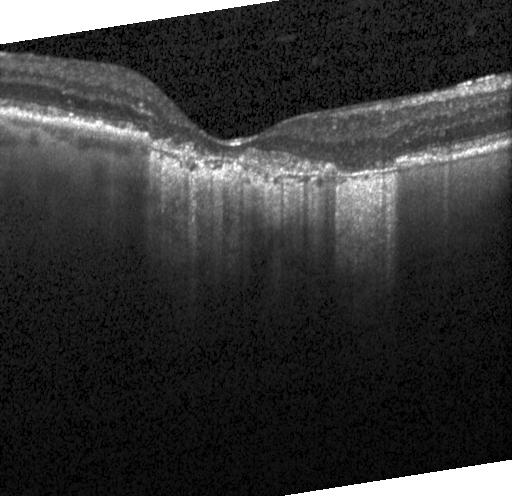 Optical coherence tomography B-scan — Diagnosis: CNV.